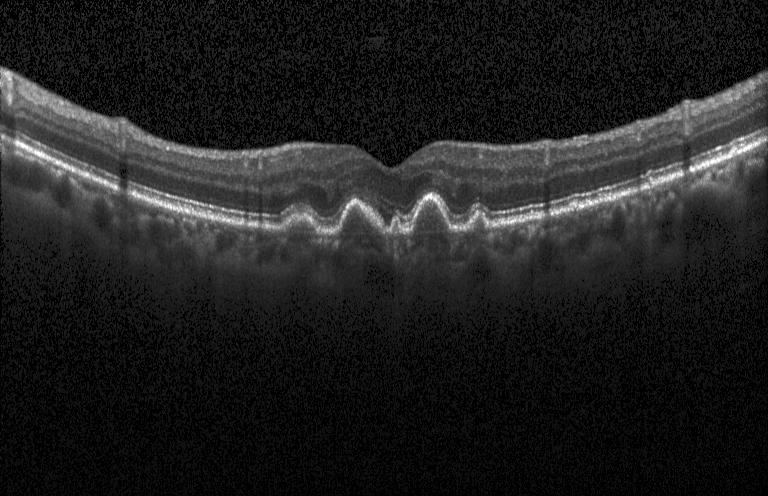 OCT finding: drusen.